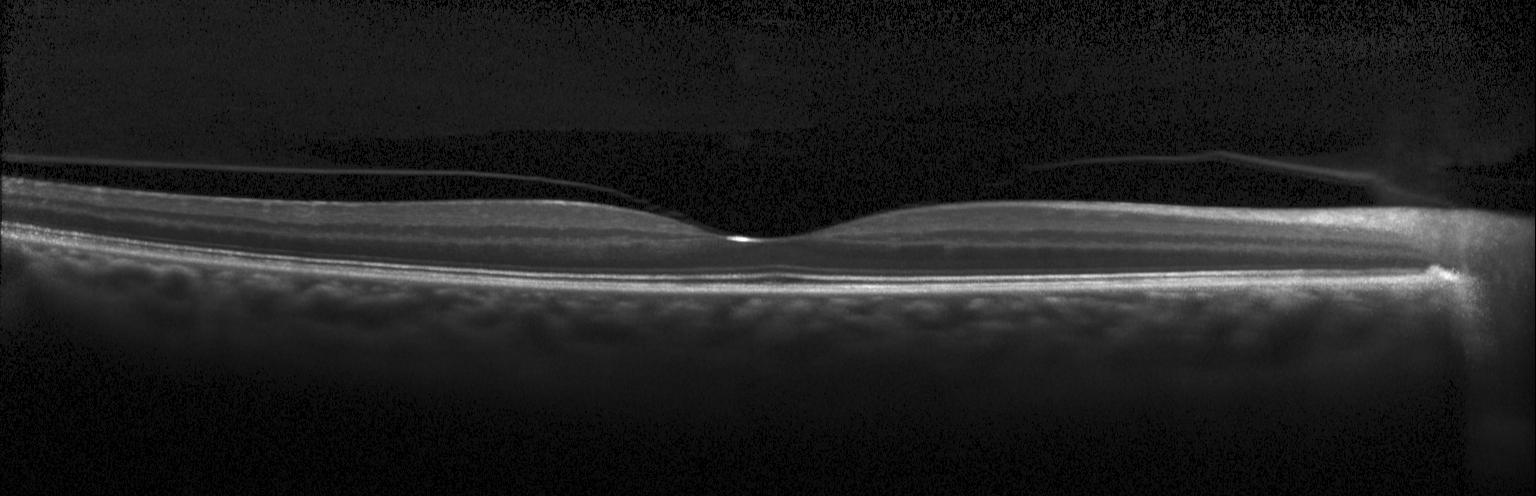

Diagnosis: neither choroidal neovascularization, diabetic macular edema, nor drusen.